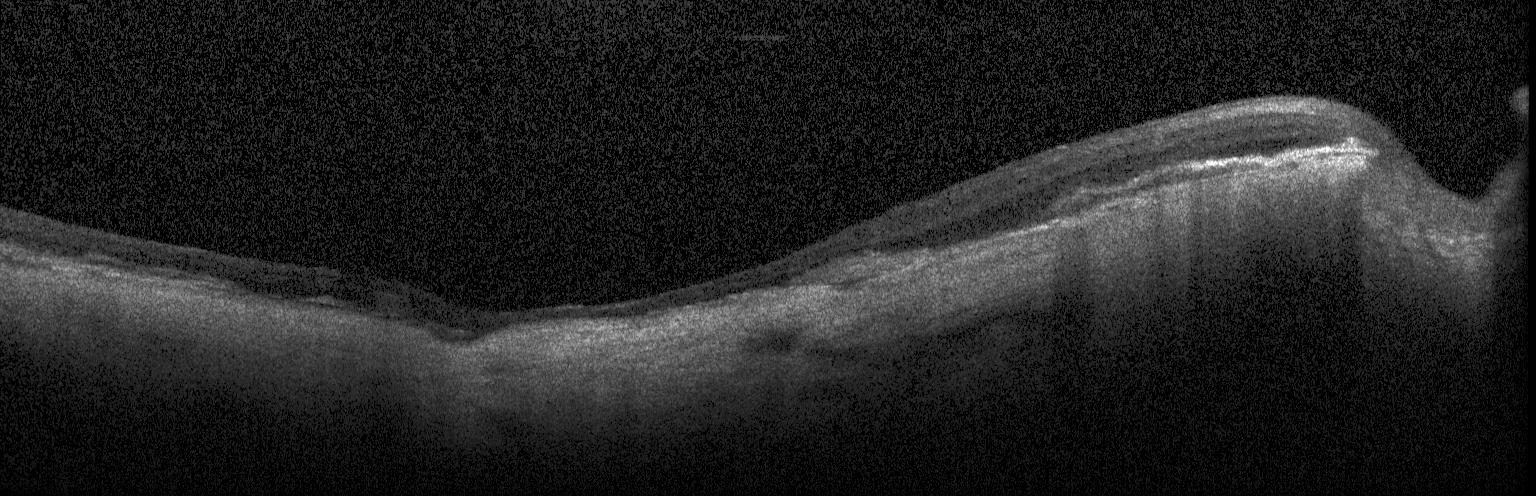

Retinal OCT cross-section. Choroidal neovascularization (CNV).